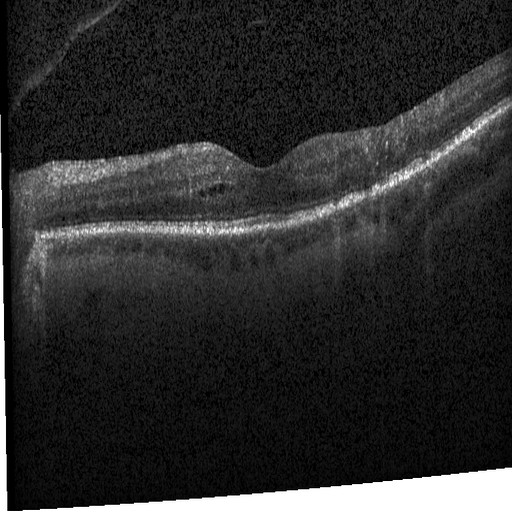
Finding: diabetic macular edema.